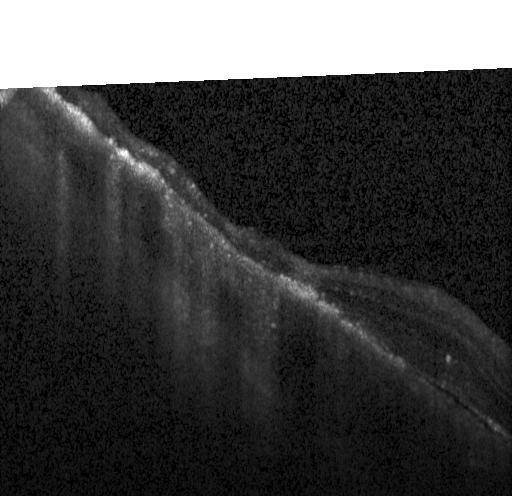

OCT line scan.
Impression: a choroidal neovascular membrane.